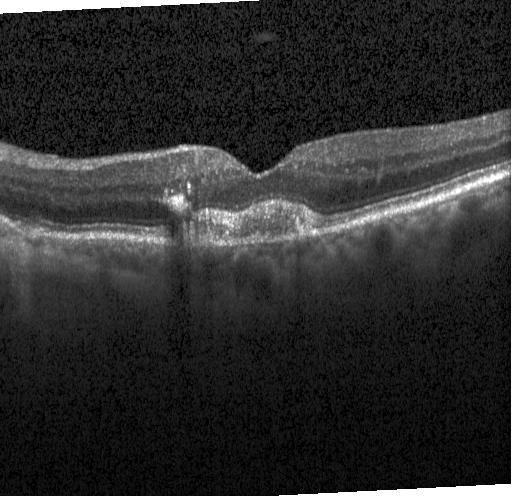
OCT finding: a choroidal neovascular membrane.